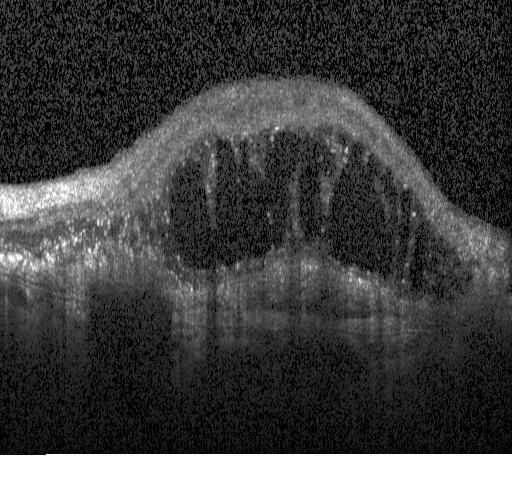

Impression: diabetic macular edema (DME).